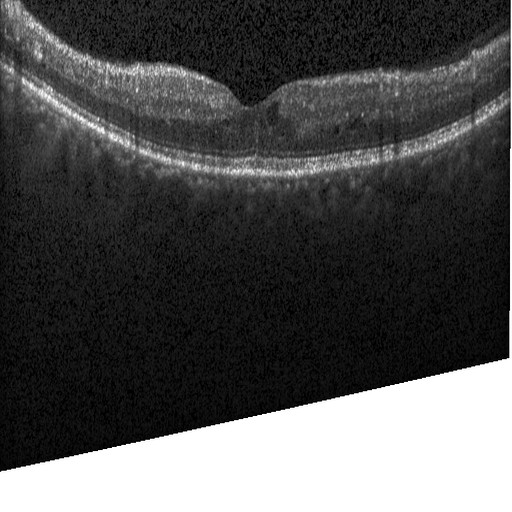

OCT line scan; fovea-centered — The scan shows DME.